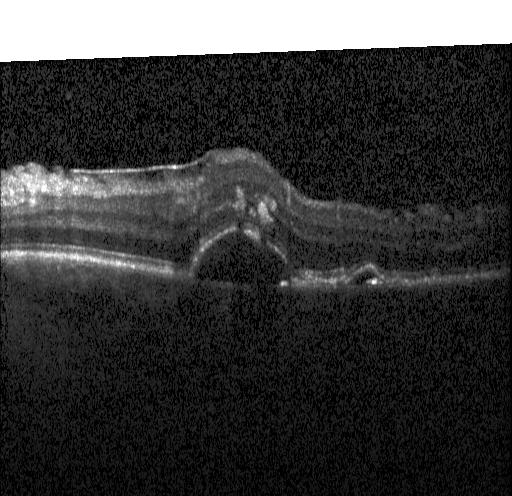

Spectral-domain OCT B-scan: a choroidal neovascular membrane.